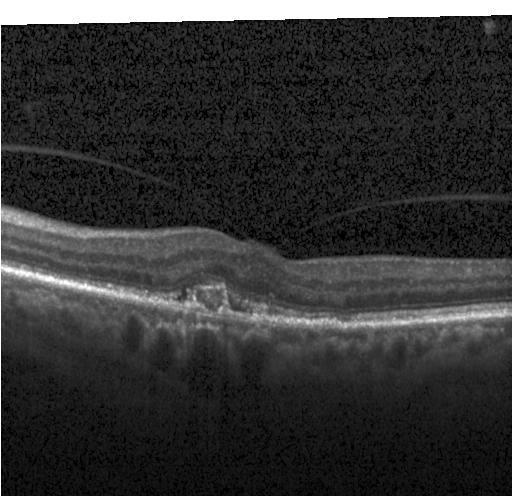 SD-OCT, acquired on a Heidelberg Spectralis, OCT B-scan. Impression: a choroidal neovascular membrane.